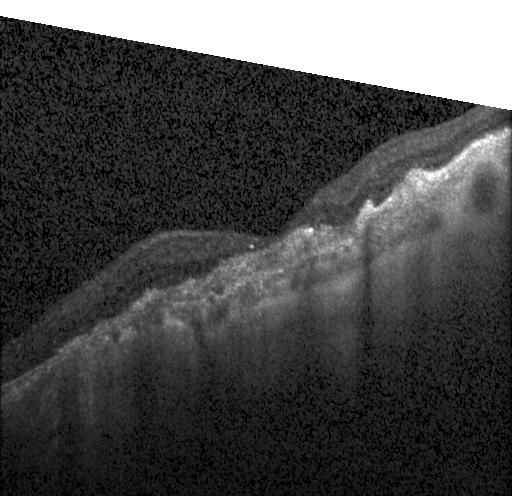
Optical coherence tomography B-scan. Spectral-domain optical coherence tomography. Through the macula
Finding: a choroidal neovascular membrane.